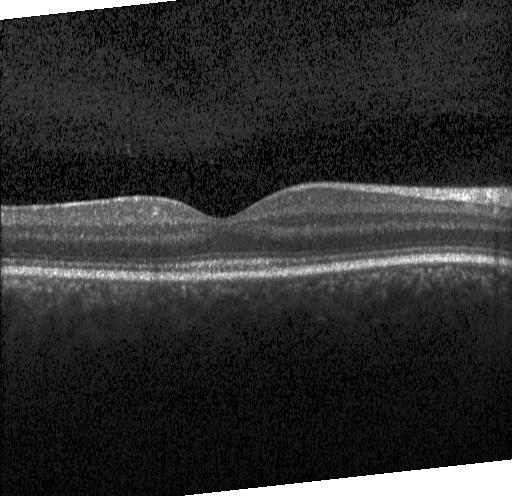

Dx: no evidence of choroidal neovascularization, diabetic macular edema, or drusen.